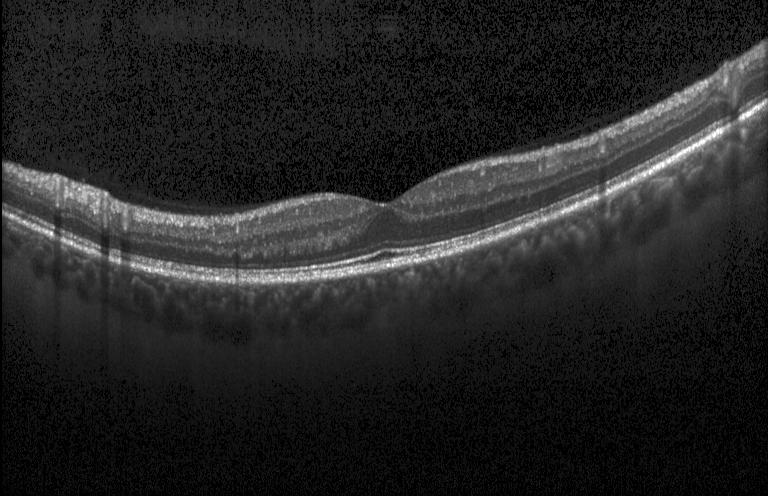 Retinal OCT cross-section showing no evidence of CNV, DME, or drusen.